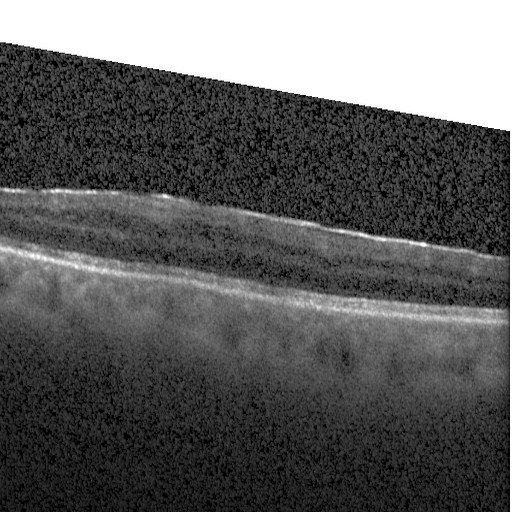
Macular OCT: diabetic macular edema (DME).